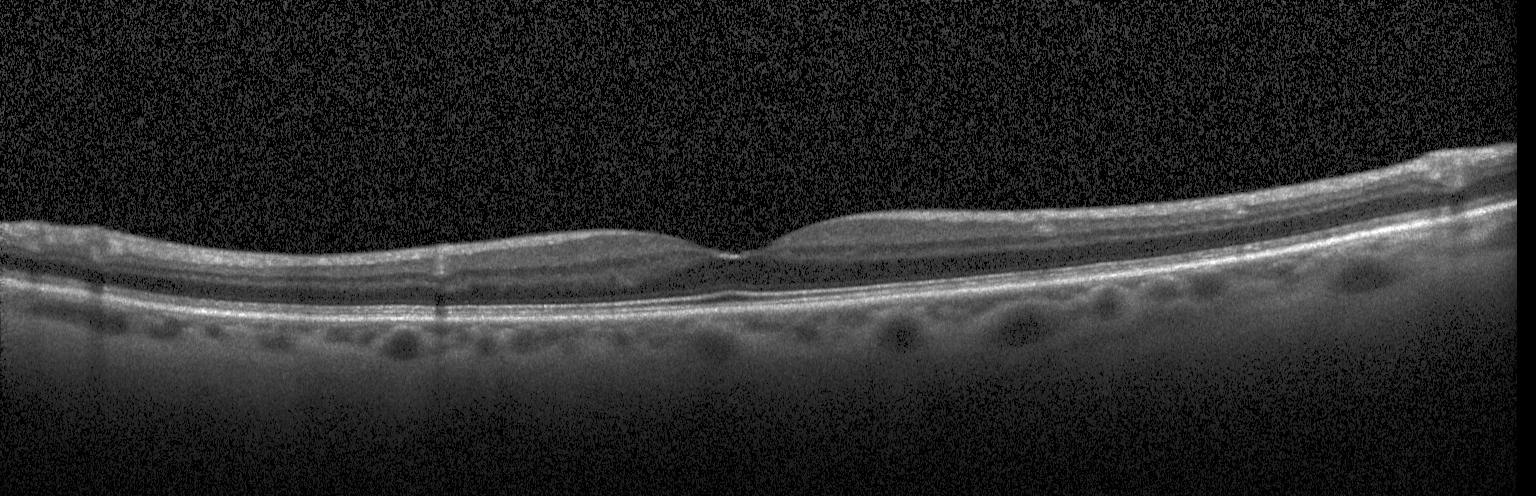 Centered on the fovea · retinal OCT B-scan.
Diagnosis: no choroidal neovascularization, no diabetic macular edema, and no drusen.